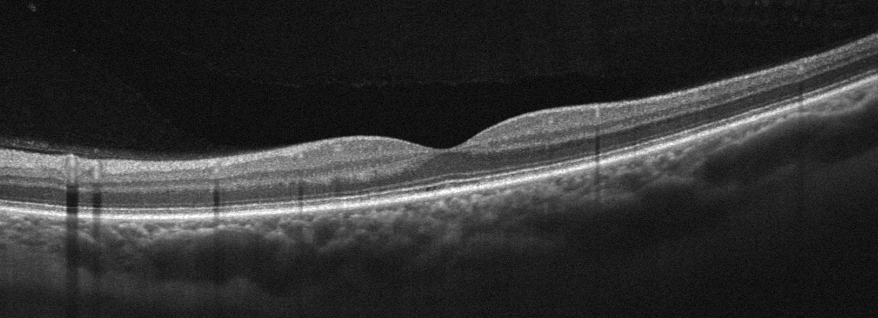
Retinal OCT cross-section showing no AMD, DME, ERM, RAO, RVO, or VID.